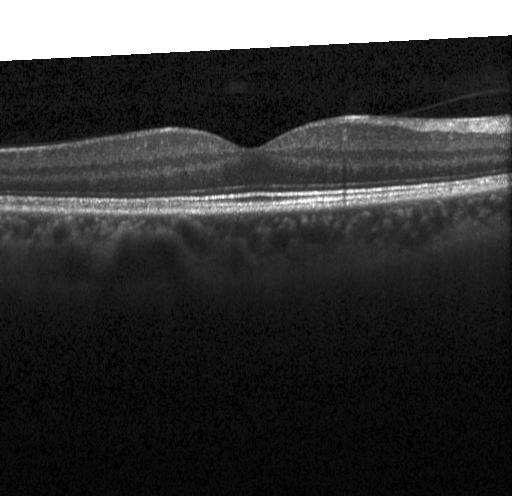

Spectral-domain optical coherence tomography; OCT line scan; instrument: Heidelberg Spectralis.
Impression: neither choroidal neovascularization, diabetic macular edema, nor drusen.